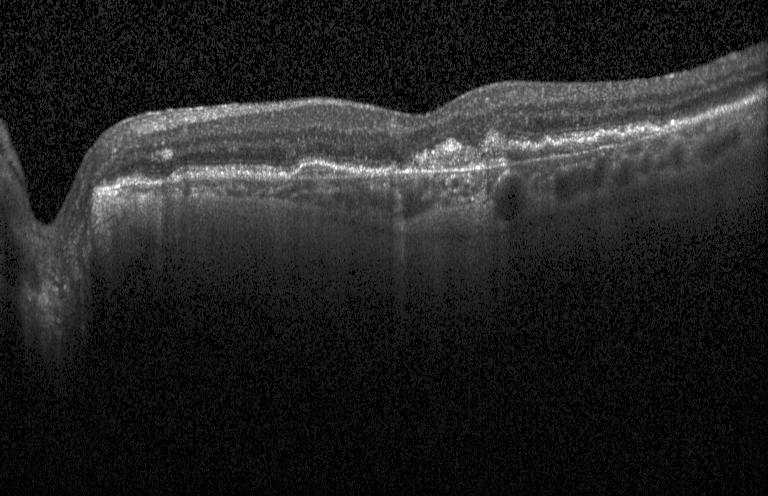
This B-scan demonstrates CNV.